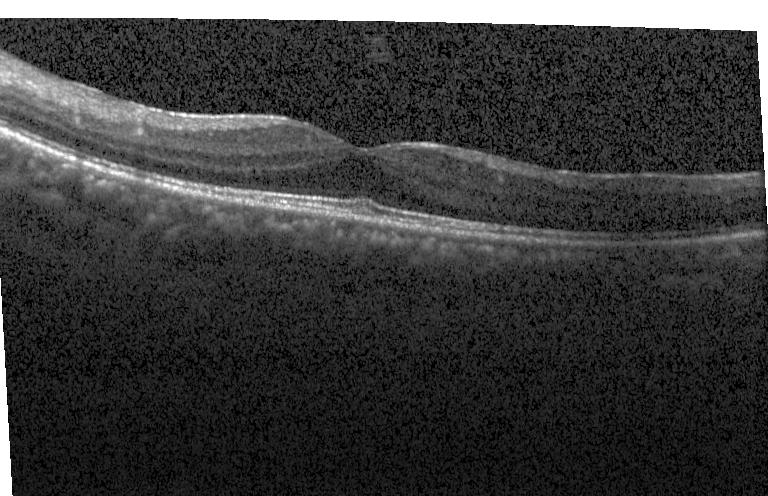
Assessment: neither CNV, DME, nor drusen.